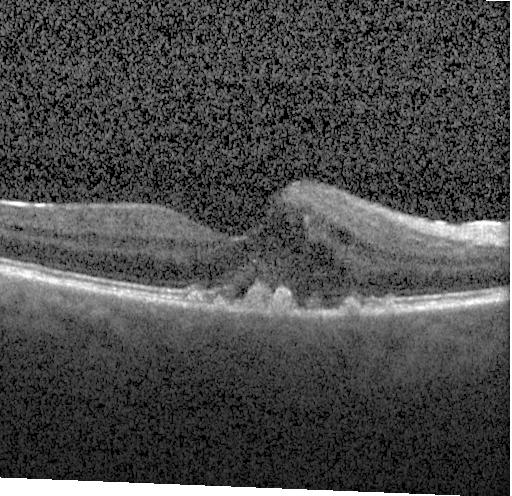 Spectral-domain optical coherence tomography · optical coherence tomography scan · horizontal scan through the fovea · instrument: Heidelberg Spectralis. Assessment: a choroidal neovascular membrane.